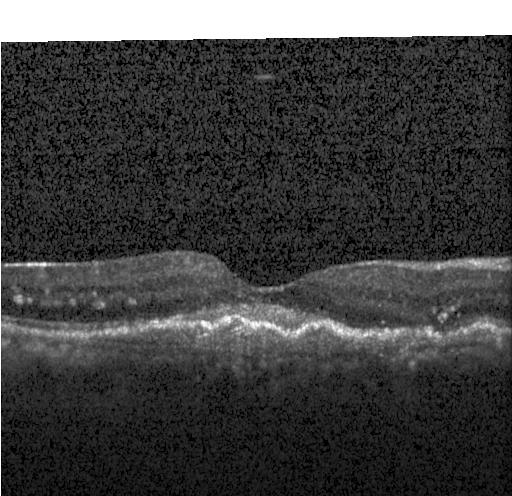

Optical coherence tomography scan.
This B-scan demonstrates CNV.